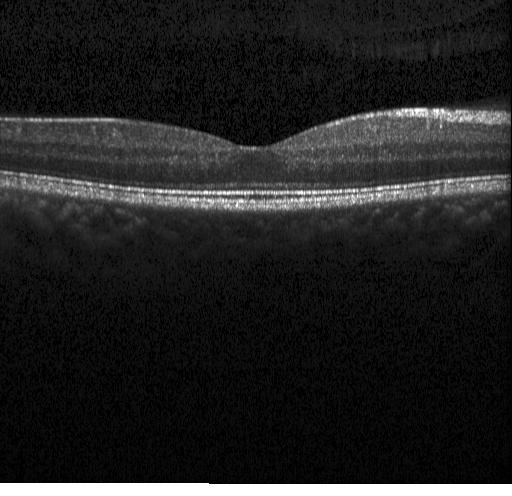
SD-OCT. Heidelberg Spectralis. OCT line scan. Fovea-centered.
Finding: no choroidal neovascularization, no diabetic macular edema, and no drusen.